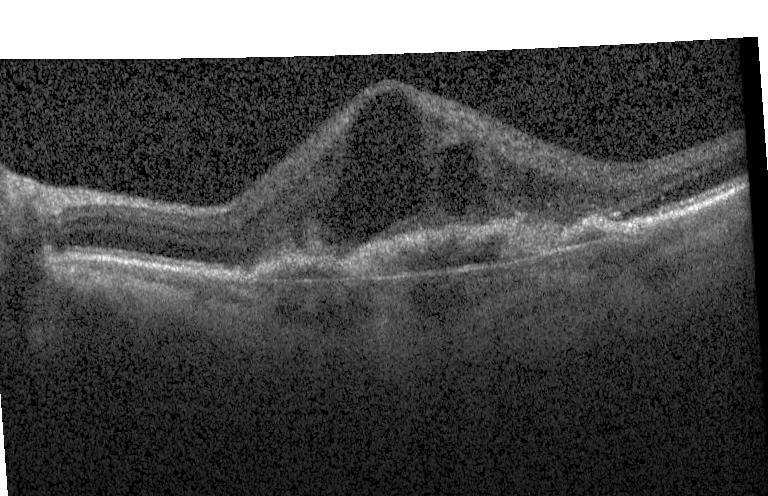 OCT scan showing choroidal neovascularization (CNV).